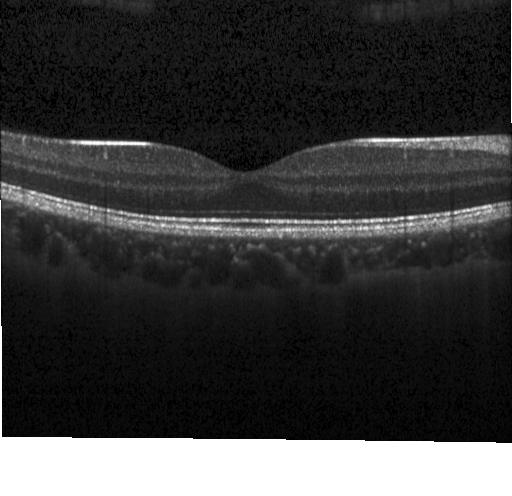
Retinal OCT cross-section showing no evidence of choroidal neovascularization, diabetic macular edema, or drusen.